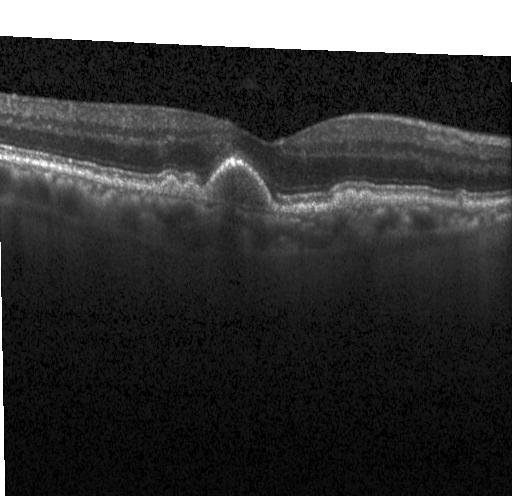
Spectral-domain OCT, optical coherence tomography scan, Heidelberg Spectralis OCT system, centered on the fovea. Assessment: sub-RPE drusenoid deposits.